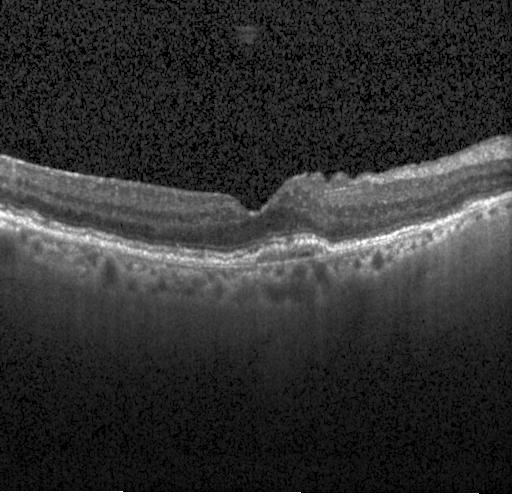

Heidelberg Spectralis. OCT line scan. Fovea-centered
Macular OCT: a choroidal neovascular membrane.